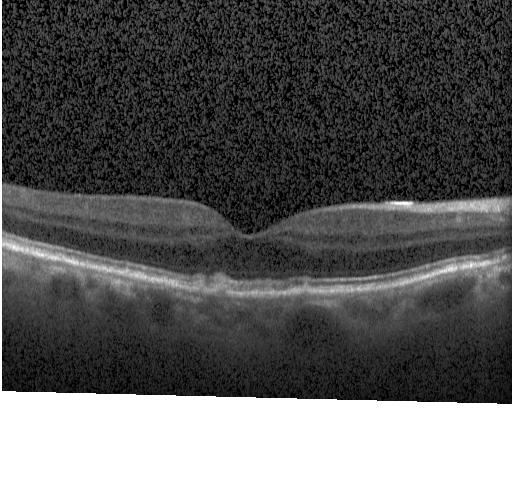
Spectral-domain OCT B-scan: multiple drusen.